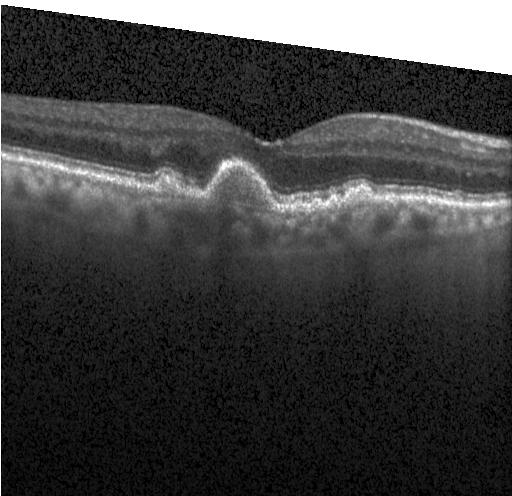
Spectral-domain optical coherence tomography. Through the macula. Optical coherence tomography B-scan. OCT finding: drusen.